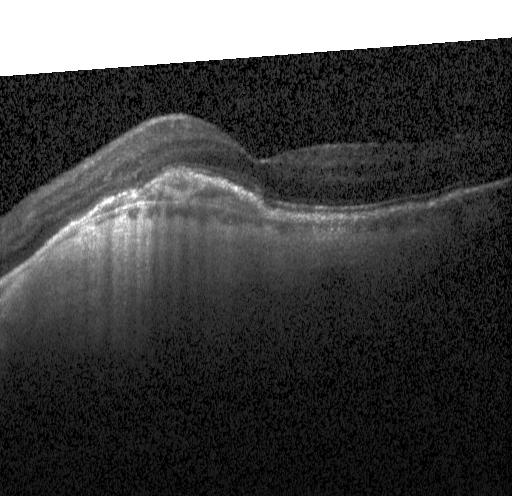

Finding: a choroidal neovascular membrane.